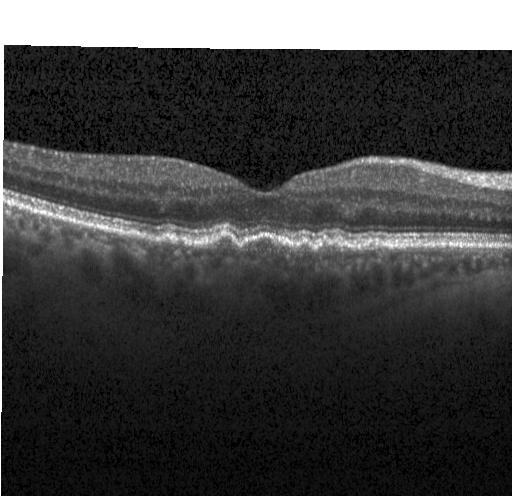

Horizontal scan through the fovea; retinal OCT B-scan; SD-OCT; Heidelberg Spectralis OCT system.
OCT finding: sub-RPE drusenoid deposits.